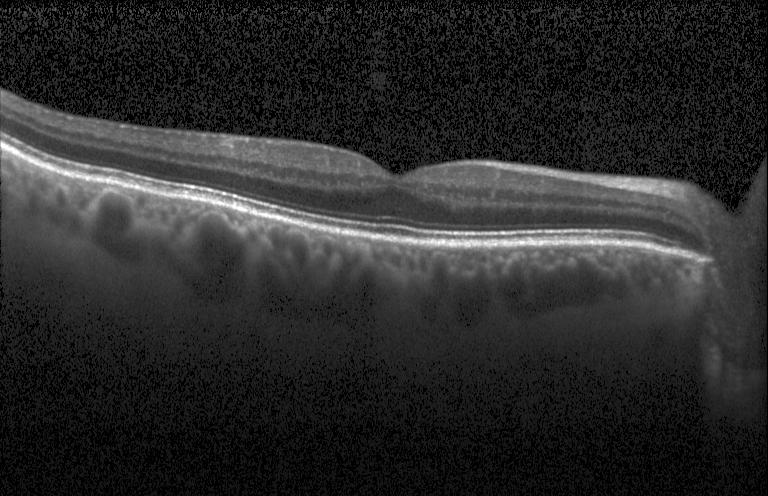
Impression: no evidence of CNV, DME, or drusen.